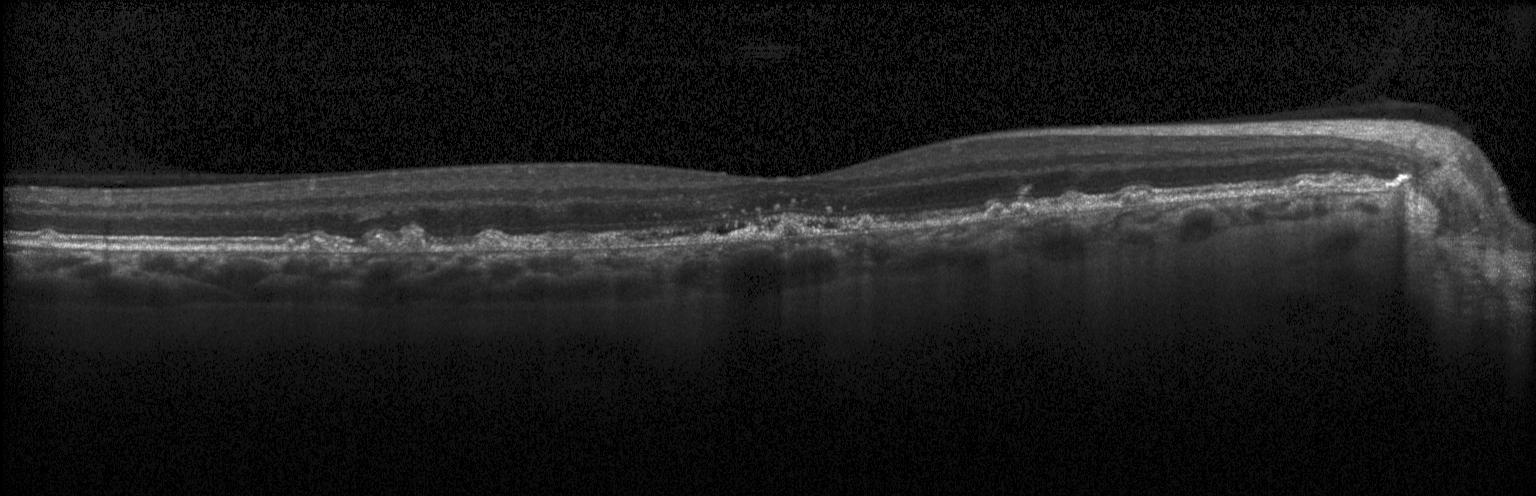

Dx: a choroidal neovascular membrane.